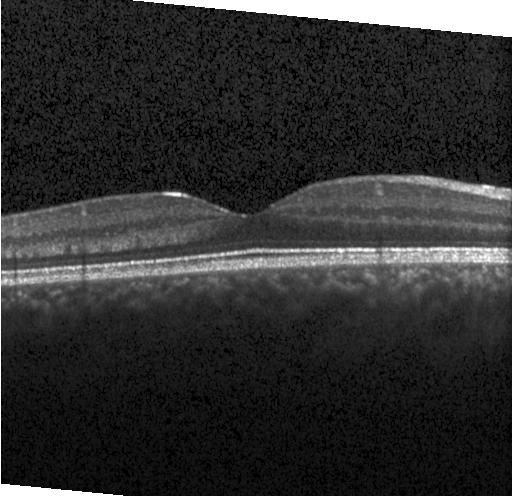
The scan shows neither choroidal neovascularization, diabetic macular edema, nor drusen.